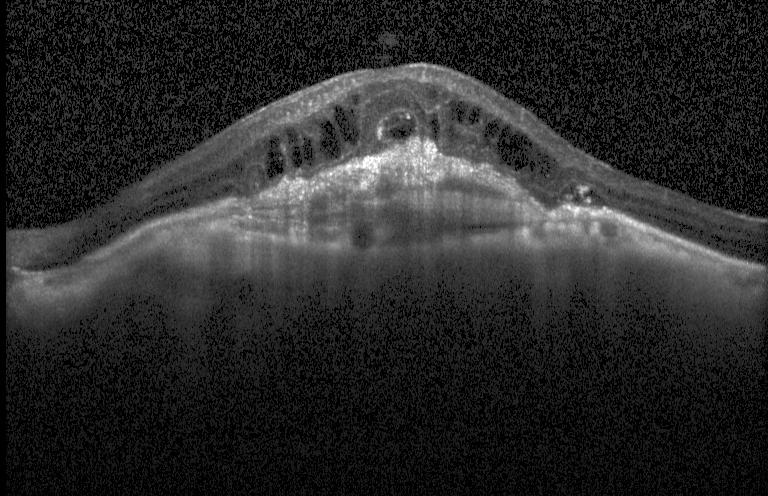
Dx: a choroidal neovascular membrane.